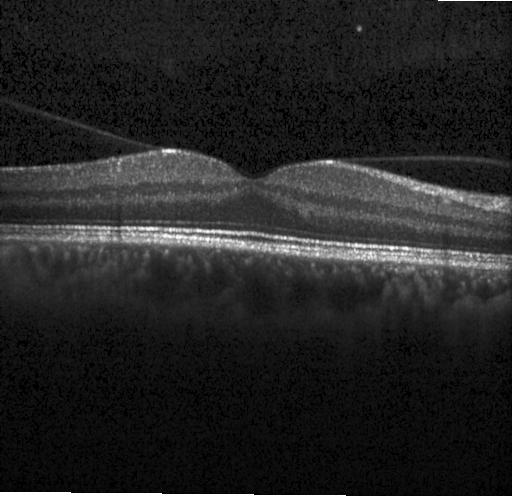 Impression: no CNV, DME, or drusen.